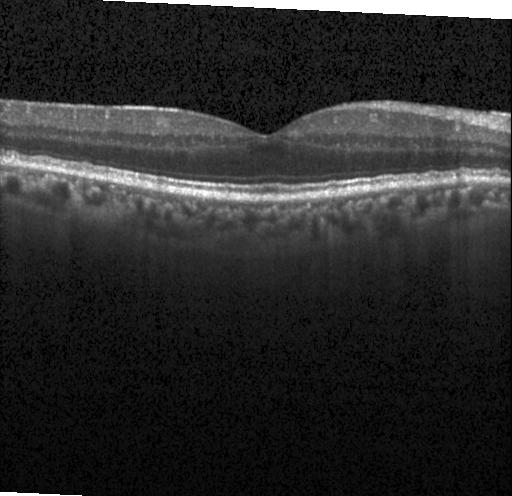
Finding: drusen.